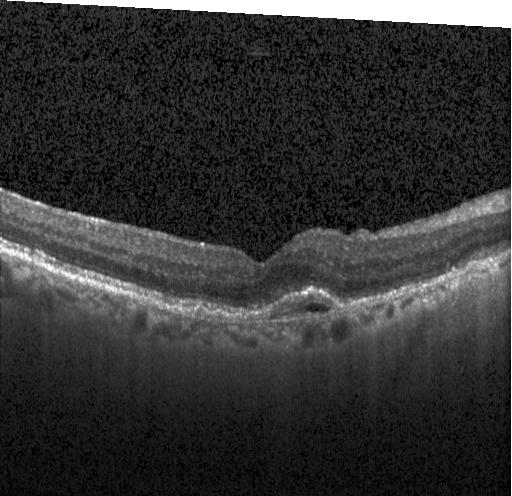
Through the macula · retinal OCT B-scan · acquired on a Heidelberg Spectralis · SD-OCT.
Diagnosis: choroidal neovascularization (CNV).